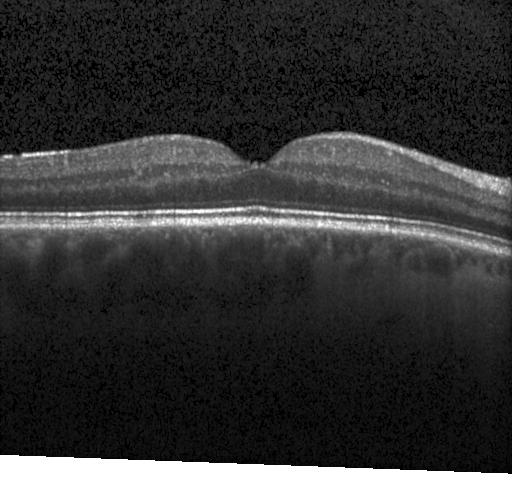
Macular OCT demonstrating no evidence of choroidal neovascularization, diabetic macular edema, or drusen.